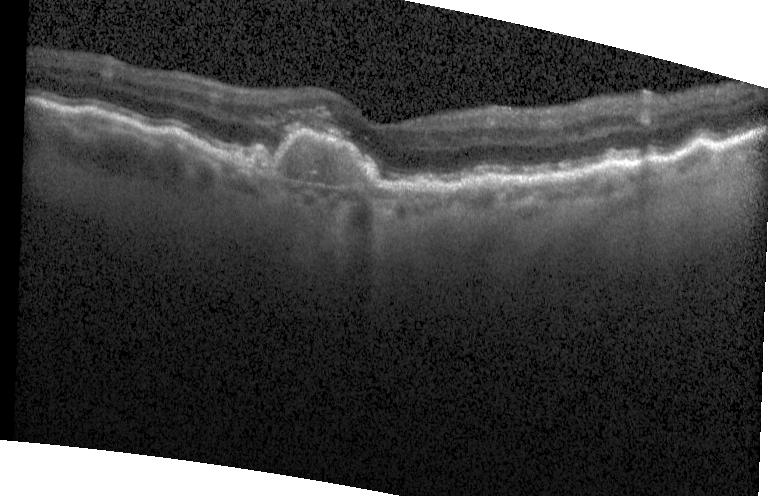
Dx: a choroidal neovascular membrane.